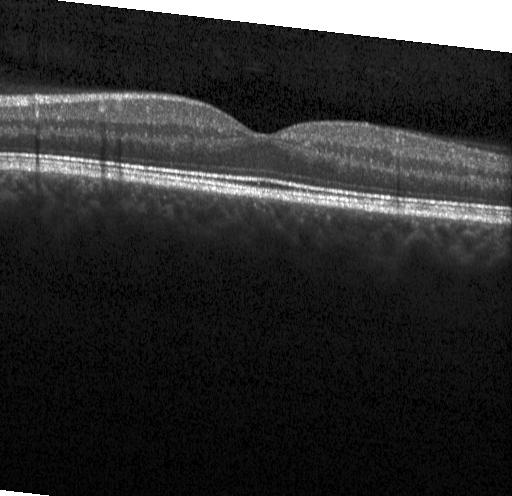 Retinal OCT B-scan.
OCT finding: no CNV, DME, or drusen.